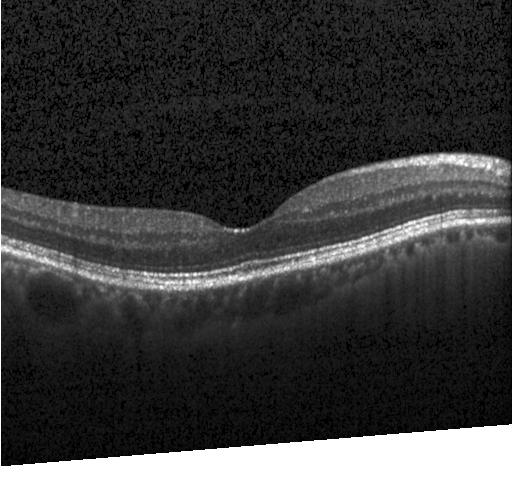

Retinal OCT B-scan. Horizontal scan through the fovea — Impression: neither choroidal neovascularization, diabetic macular edema, nor drusen.